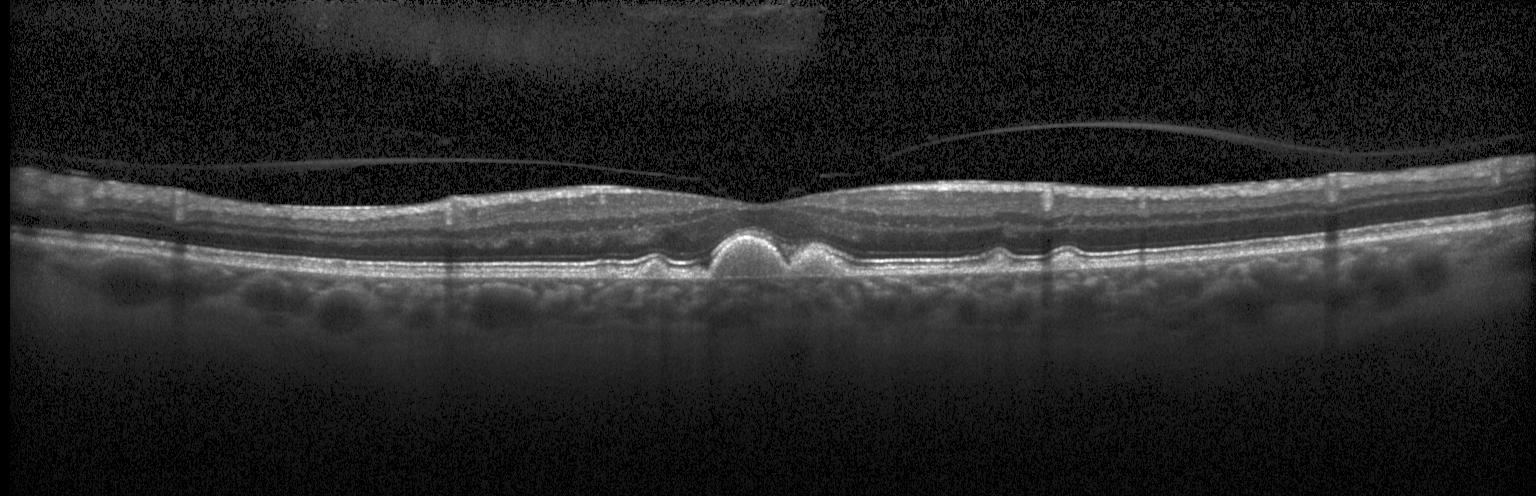 Impression: sub-RPE drusenoid deposits.